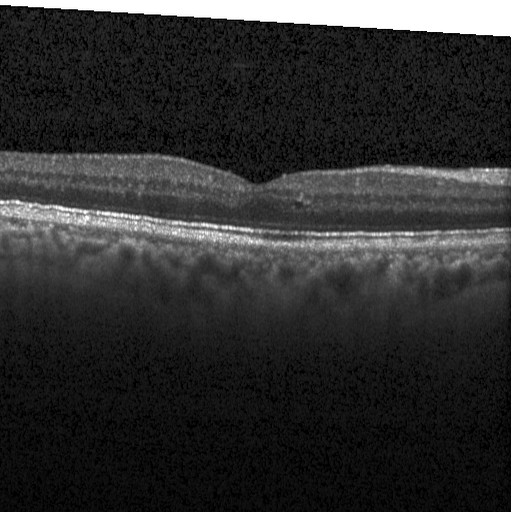

Optical coherence tomography scan — Finding: diabetic macular edema.